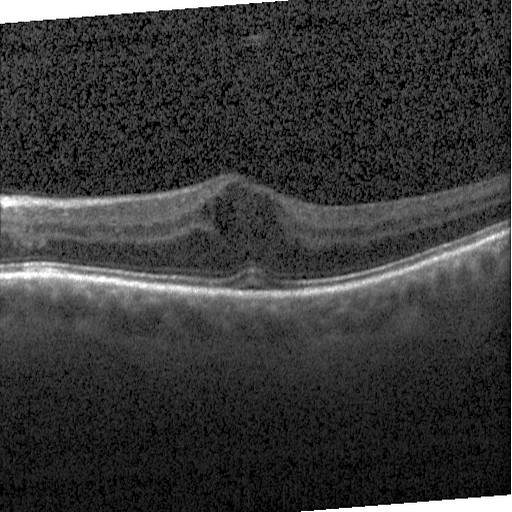
SD-OCT; optical coherence tomography scan; macular scan. Assessment: diabetic macular edema (DME).